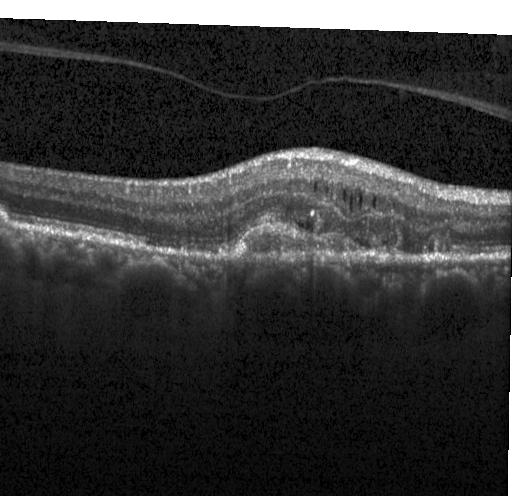
Heidelberg Spectralis; macular scan; spectral-domain OCT; optical coherence tomography B-scan
This B-scan demonstrates a choroidal neovascular membrane.